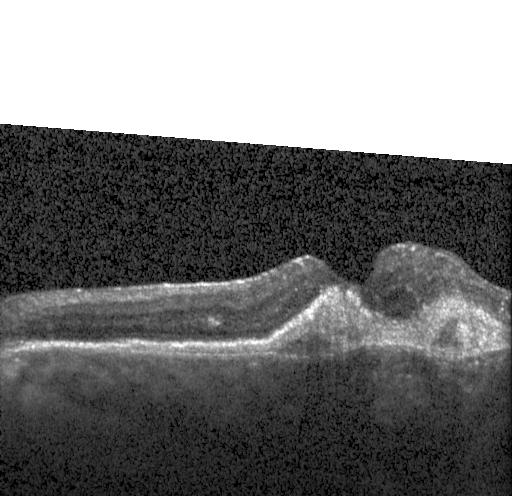

Through the macula. Optical coherence tomography B-scan. SD-OCT
Macular OCT: choroidal neovascularization.